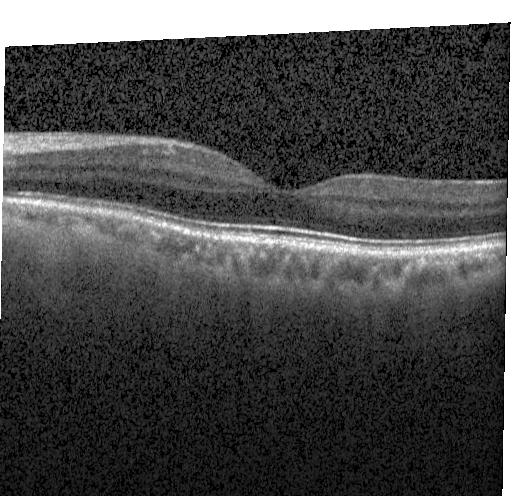

Optical coherence tomography B-scan, Heidelberg Spectralis. The scan shows neither CNV, DME, nor drusen.